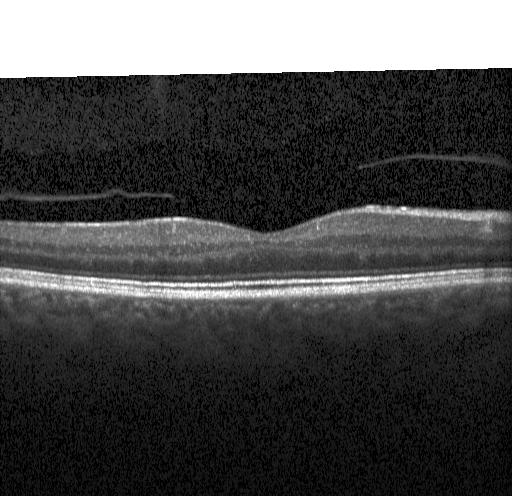 The scan shows no choroidal neovascularization, no diabetic macular edema, and no drusen.